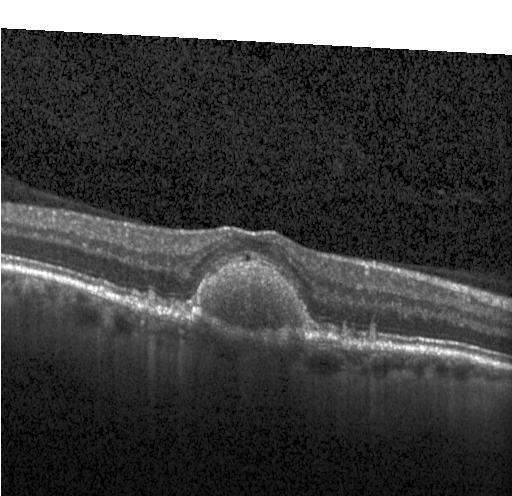
Acquired on a Heidelberg Spectralis. Retinal OCT B-scan.
Assessment: a choroidal neovascular membrane.